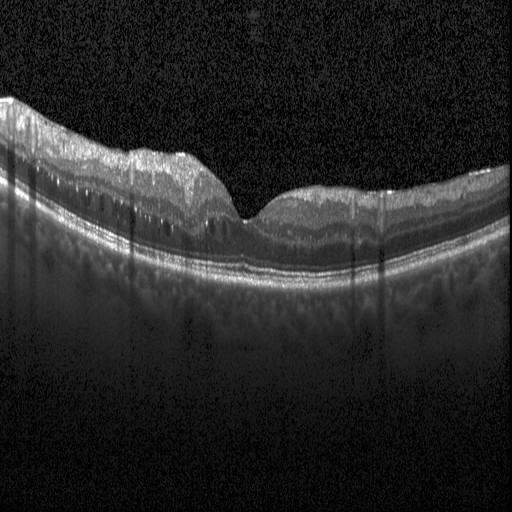

Optical coherence tomography scan.
Dx: diabetic macular edema (DME).